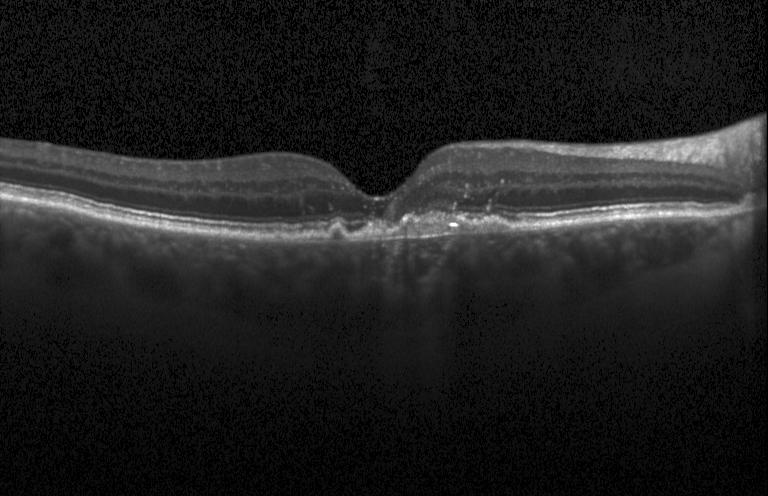
Spectral-domain optical coherence tomography, acquired on a Heidelberg Spectralis, optical coherence tomography B-scan, centered on the fovea.
Diagnosis: a choroidal neovascular membrane.